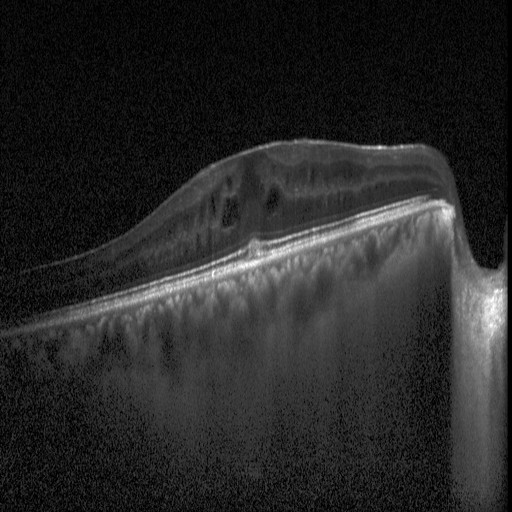
OCT finding: DME.